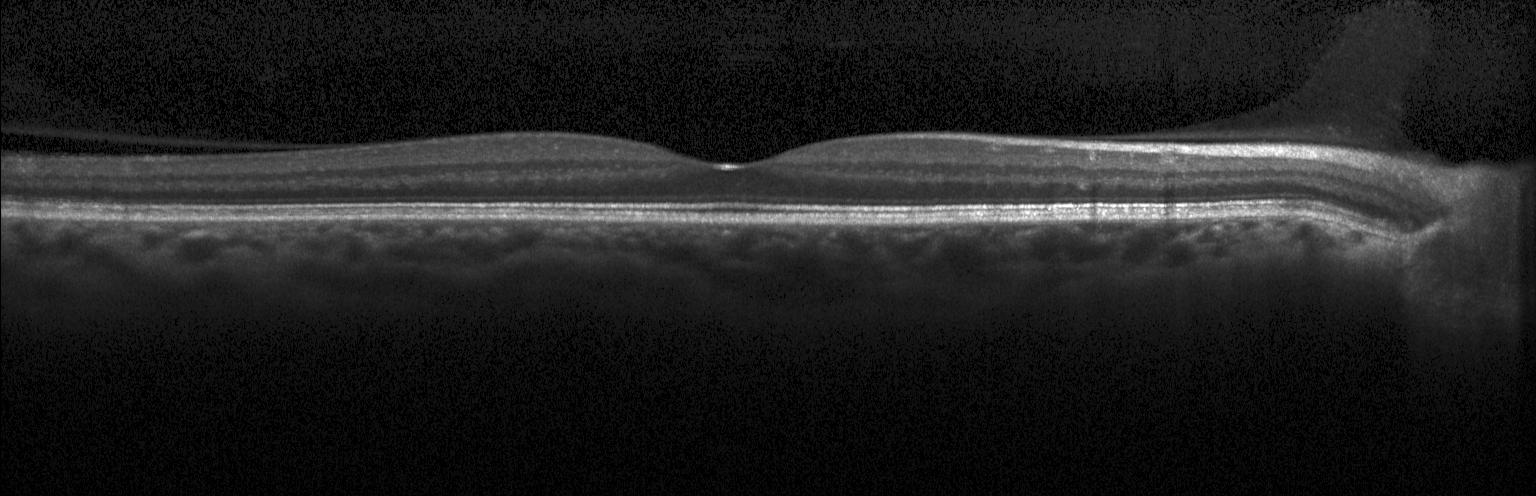
Spectral-domain OCT B-scan: no choroidal neovascularization, diabetic macular edema, or drusen.